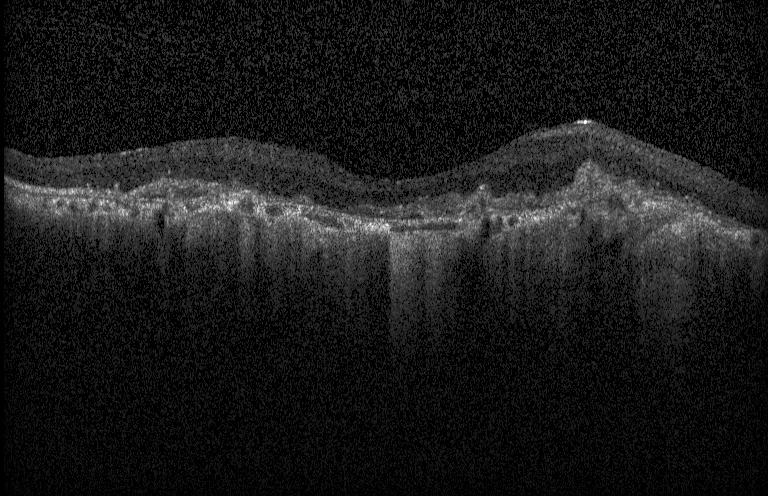
Macular scan, acquired on a Heidelberg Spectralis, optical coherence tomography B-scan, SD-OCT.
Dx: a choroidal neovascular membrane.